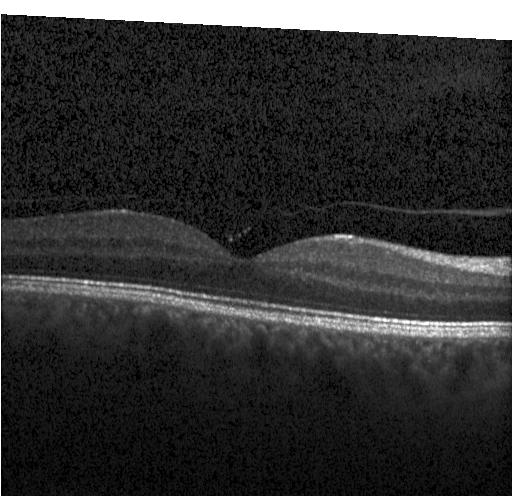

OCT B-scan. Through the macula. Finding: no choroidal neovascularization, diabetic macular edema, or drusen.